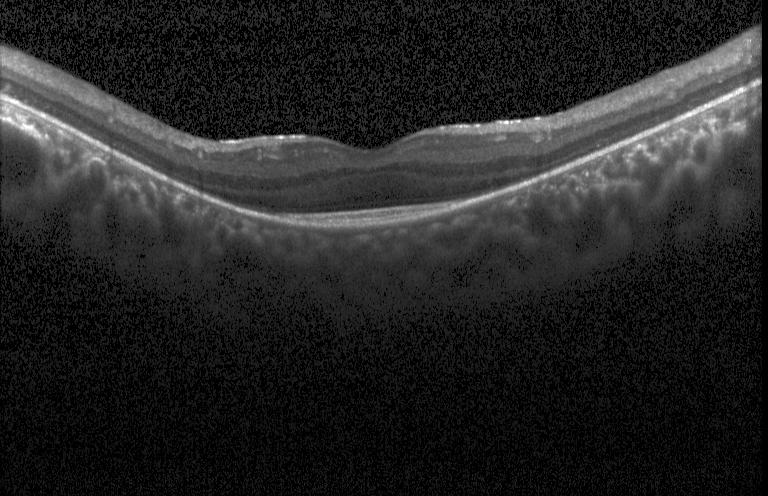

Fovea-centered. Instrument: Heidelberg Spectralis. Spectral-domain OCT. OCT line scan
This B-scan demonstrates neither choroidal neovascularization, diabetic macular edema, nor drusen.